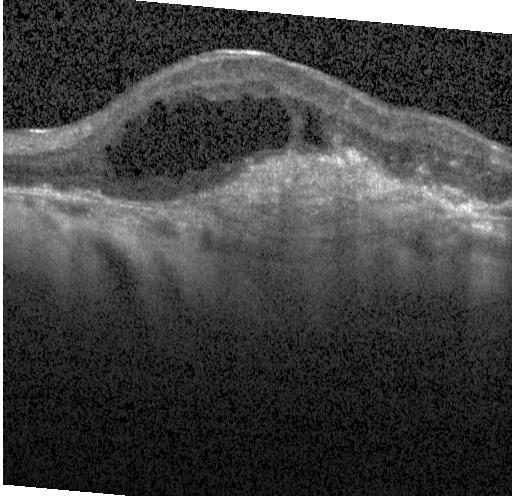 Optical coherence tomography B-scan.
Impression: choroidal neovascularization.